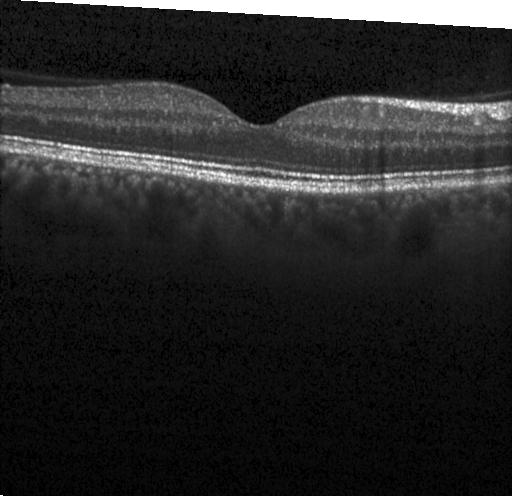 Spectral-domain OCT · OCT B-scan · Heidelberg Spectralis OCT system
Diagnosis: neither choroidal neovascularization, diabetic macular edema, nor drusen.